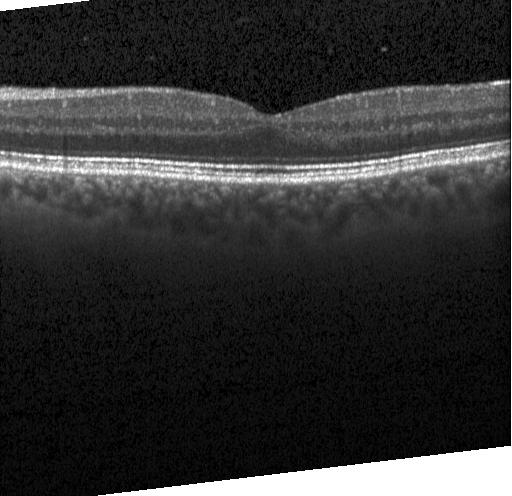

SD-OCT; Heidelberg Spectralis; retinal OCT B-scan; centered on the fovea. Finding: no choroidal neovascularization, diabetic macular edema, or drusen.